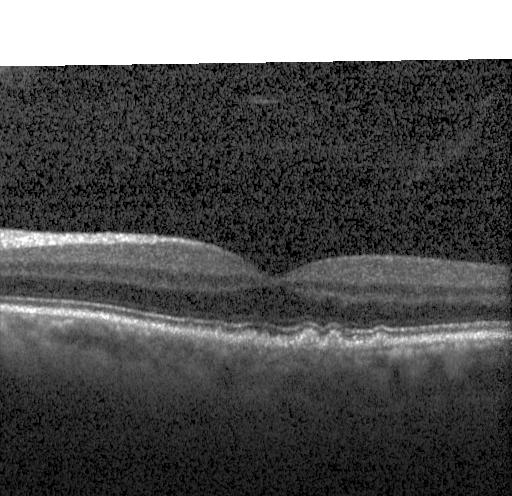
SD-OCT; OCT line scan; horizontal scan through the fovea.
Dx: sub-RPE drusenoid deposits.